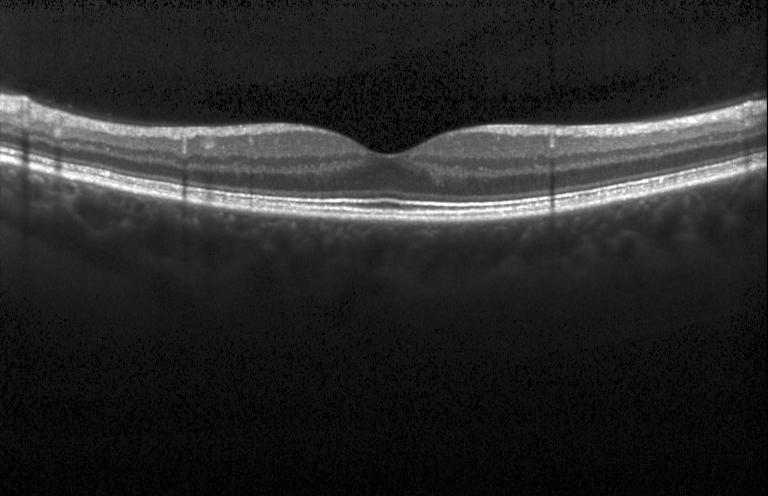

Heidelberg Spectralis, spectral-domain optical coherence tomography, optical coherence tomography scan, through the macula — Finding: no choroidal neovascularization, diabetic macular edema, or drusen.